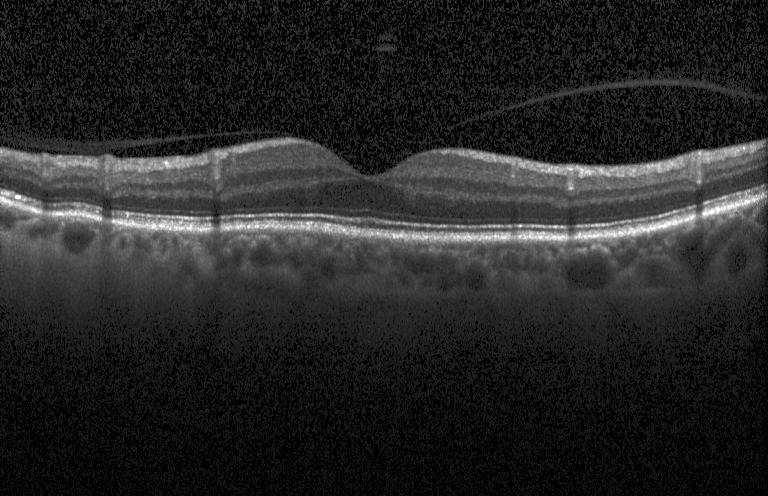
Retinal OCT B-scan. Fovea-centered
No choroidal neovascularization, diabetic macular edema, or drusen.